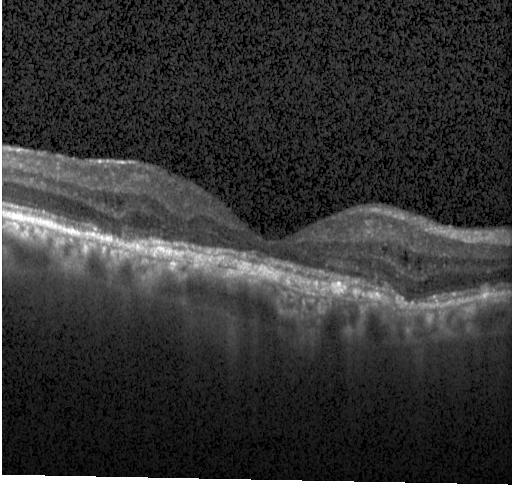
Heidelberg Spectralis OCT system; OCT B-scan; spectral-domain optical coherence tomography. Impression: choroidal neovascularization.